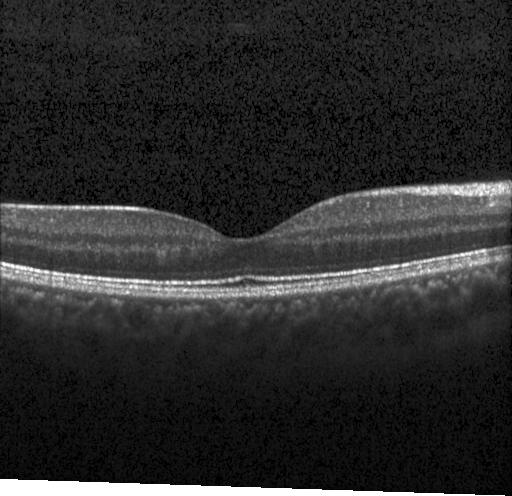

Instrument: Heidelberg Spectralis, optical coherence tomography B-scan — This B-scan demonstrates no choroidal neovascularization, diabetic macular edema, or drusen.